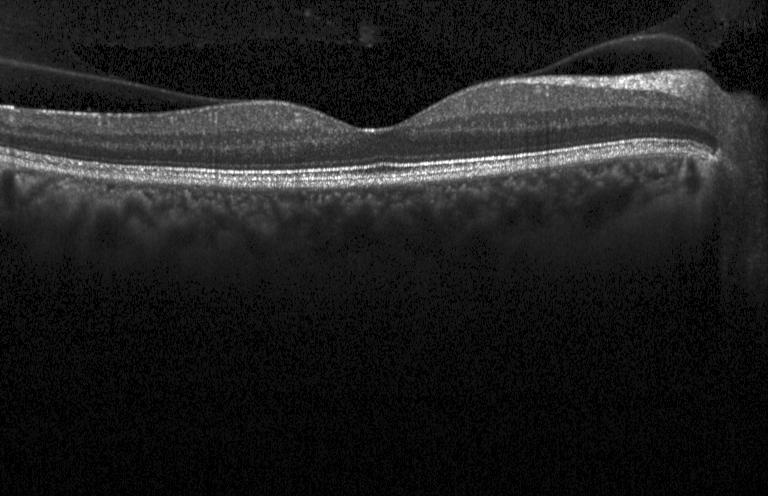 Optical coherence tomography B-scan — OCT finding: no choroidal neovascularization, no diabetic macular edema, and no drusen.